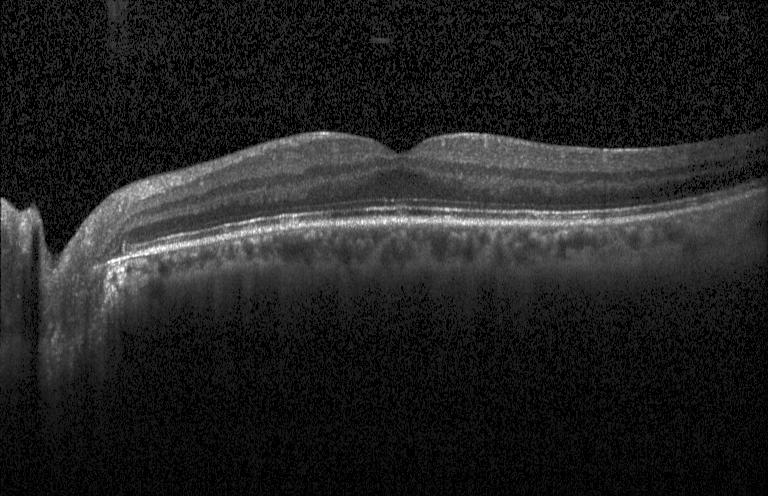 Retinal OCT B-scan, macular scan, spectral-domain OCT — Finding: neither choroidal neovascularization, diabetic macular edema, nor drusen.